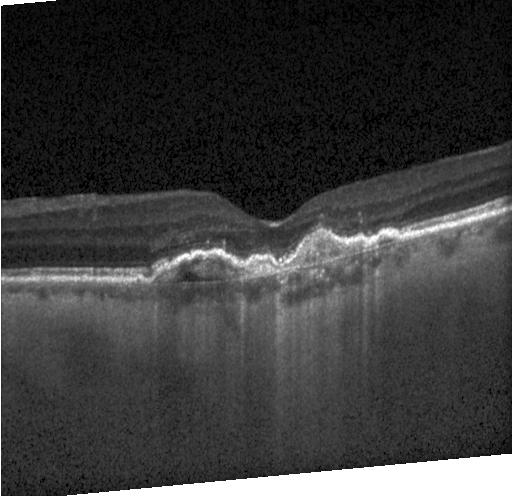 Finding: choroidal neovascularization (CNV).